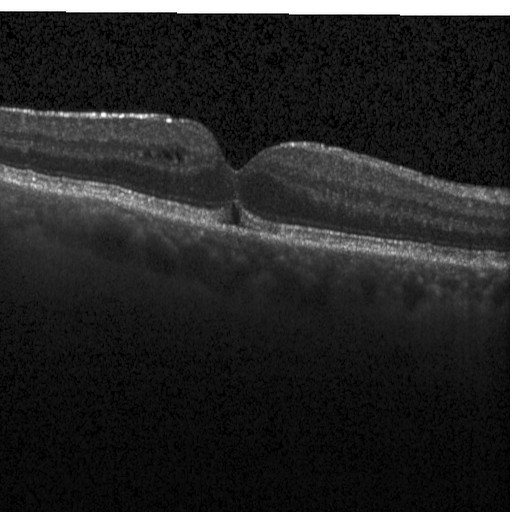 This B-scan demonstrates diabetic macular edema (DME).